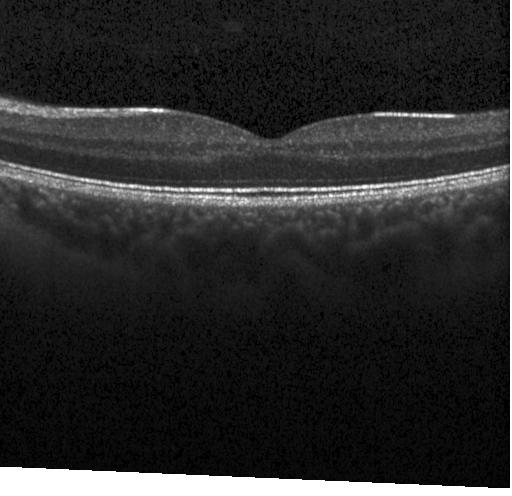

OCT line scan
Macular OCT: no choroidal neovascularization, no diabetic macular edema, and no drusen.